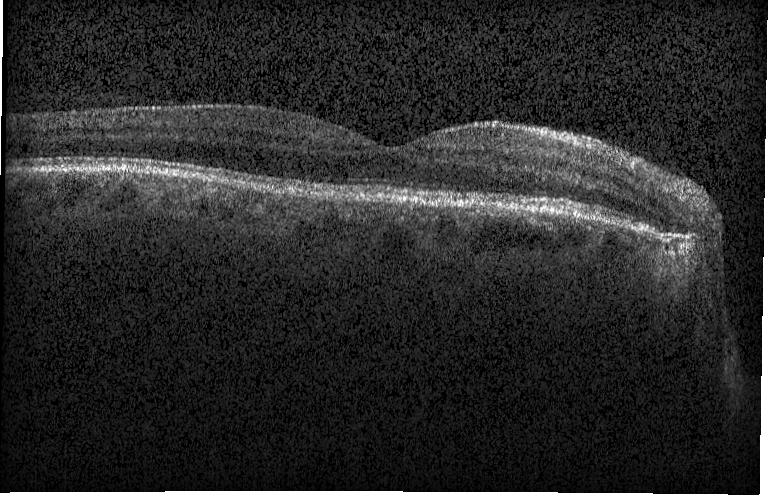

Dx: no choroidal neovascularization, diabetic macular edema, or drusen.